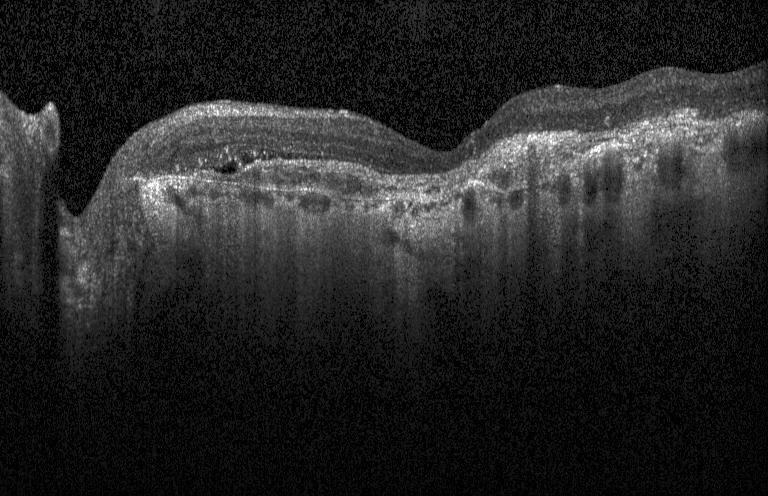 Assessment: CNV.